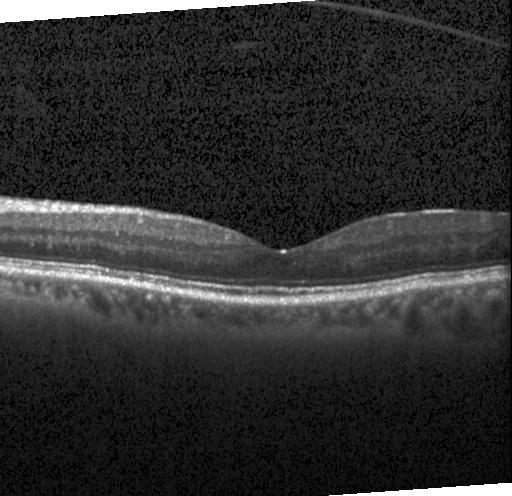

Spectral-domain optical coherence tomography, fovea-centered, retinal OCT B-scan
This B-scan demonstrates no CNV, DME, or drusen.